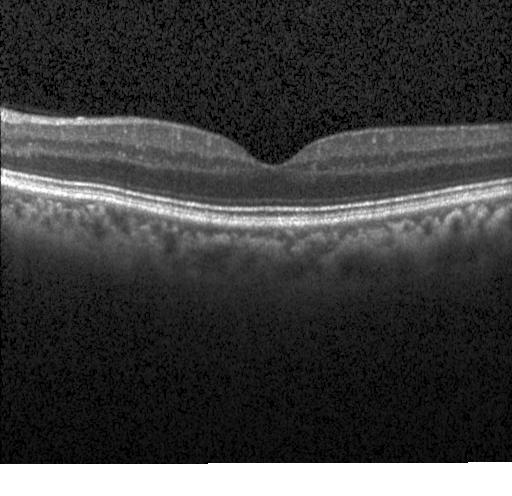 Heidelberg Spectralis OCT system, retinal OCT cross-section. Finding: neither choroidal neovascularization, diabetic macular edema, nor drusen.